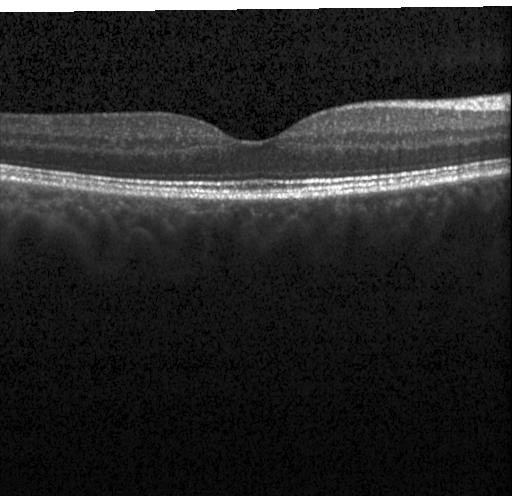
Retinal OCT cross-section — Impression: no CNV, DME, or drusen.